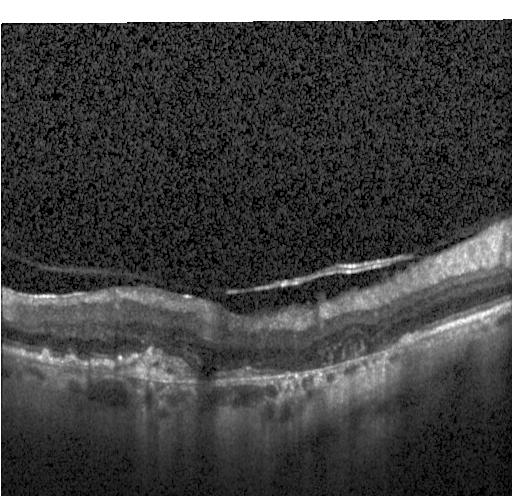

OCT line scan; spectral-domain OCT. OCT finding: a choroidal neovascular membrane.